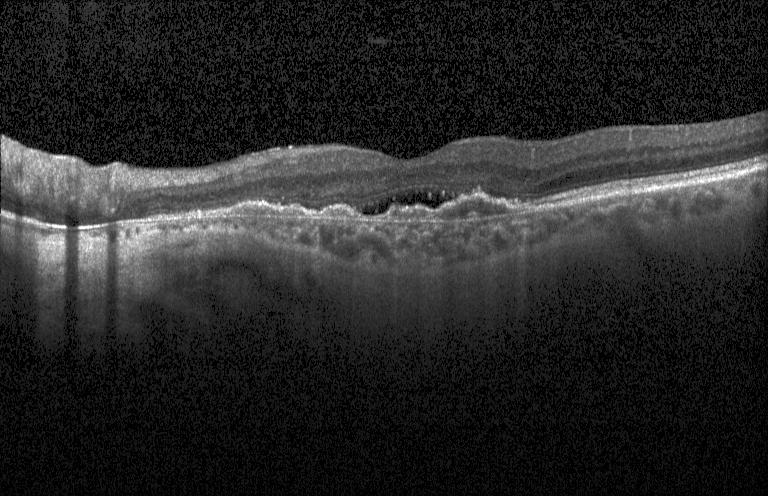 Macular scan; retinal OCT B-scan; spectral-domain optical coherence tomography — Macular OCT: a choroidal neovascular membrane.